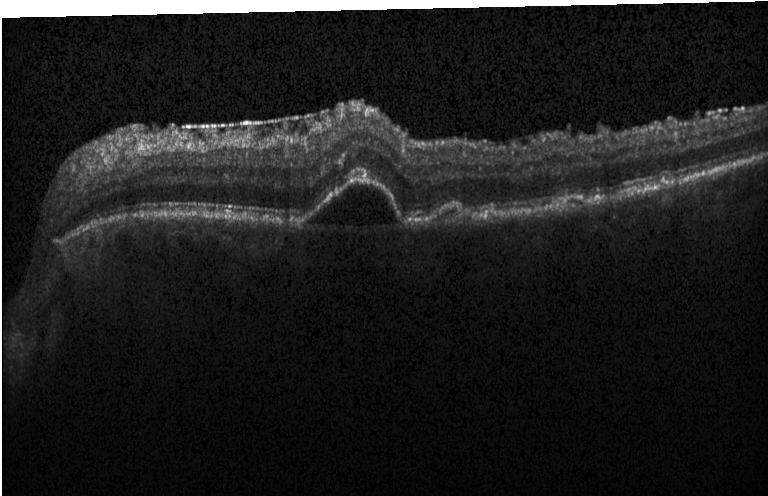 Diagnosis: choroidal neovascularization (CNV).